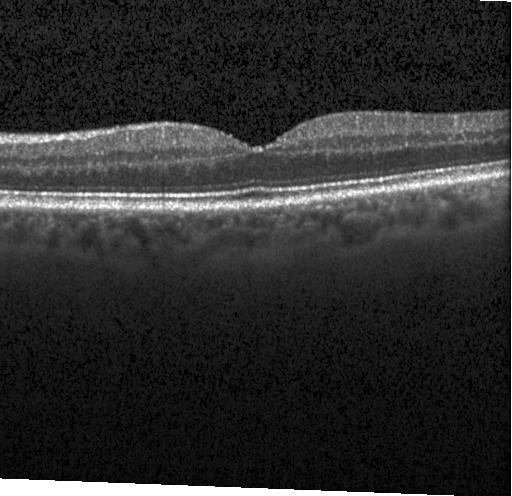 Retinal OCT B-scan. Finding: no choroidal neovascularization, no diabetic macular edema, and no drusen.